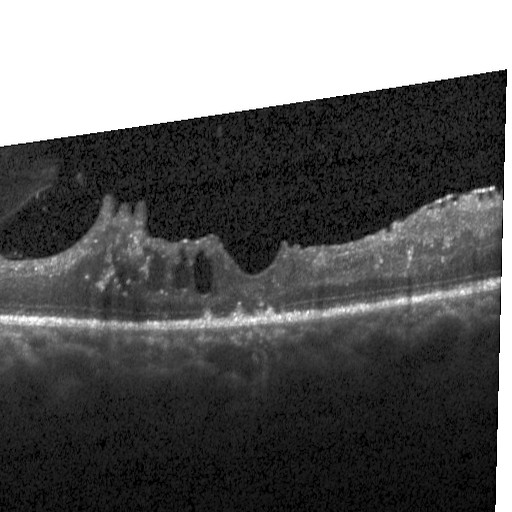
Impression: DME.